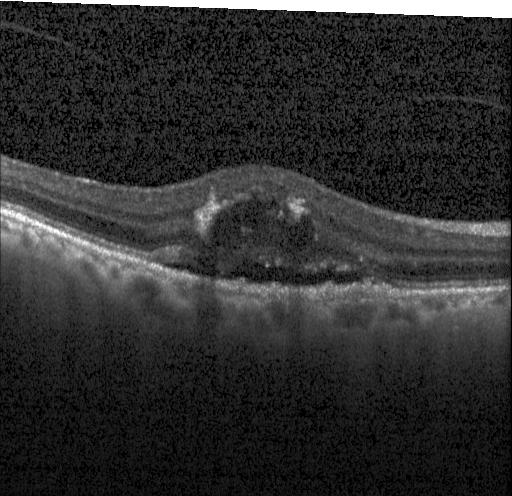 SD-OCT, retinal OCT cross-section — Finding: CNV.